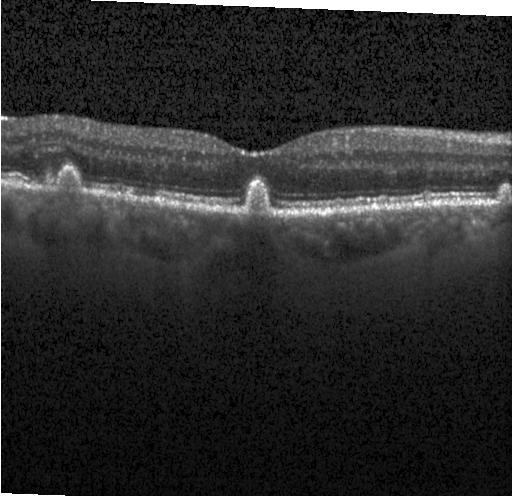 OCT line scan. Acquired on a Heidelberg Spectralis. Macular scan. The scan shows sub-RPE drusenoid deposits.